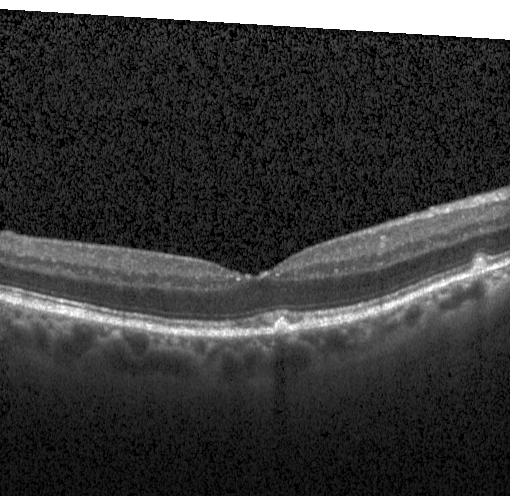

Optical coherence tomography B-scan
Finding: sub-RPE drusenoid deposits.